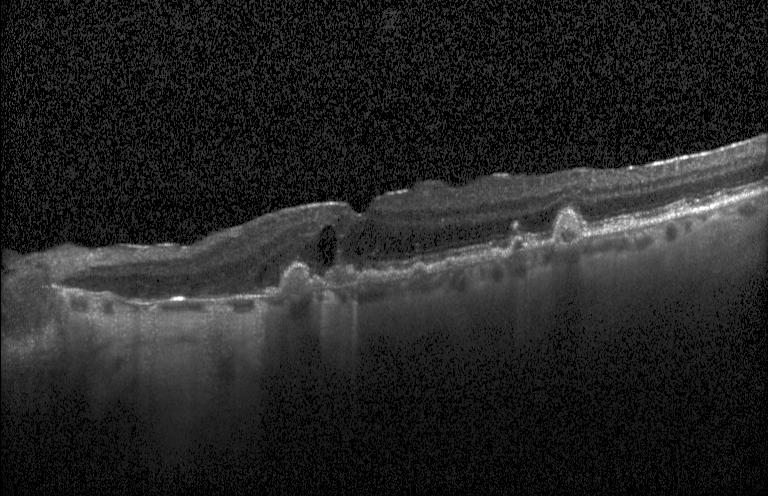 Impression: CNV.